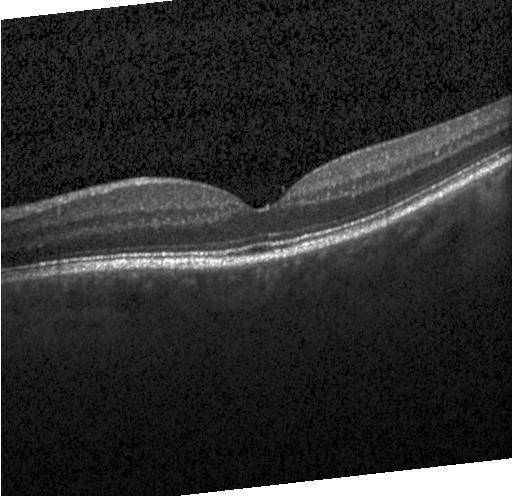
Spectral-domain OCT, OCT B-scan, centered on the fovea, Heidelberg Spectralis — Impression: no evidence of choroidal neovascularization, diabetic macular edema, or drusen.